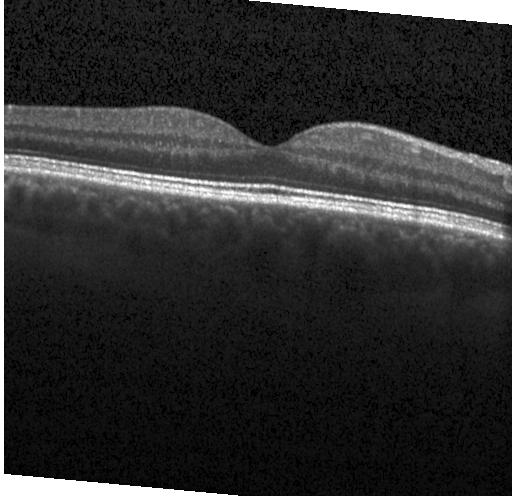
Retinal OCT cross-section
Finding: no evidence of CNV, DME, or drusen.